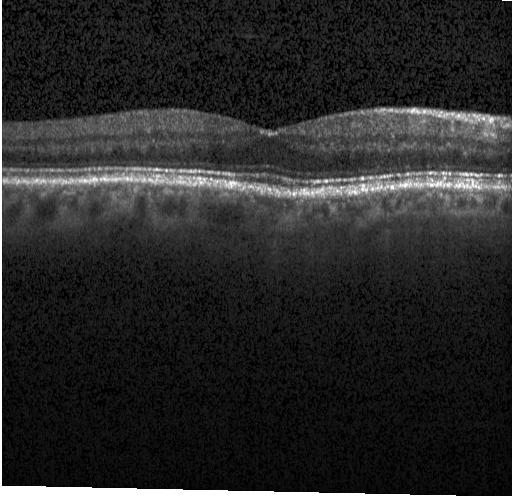 Heidelberg Spectralis, retinal OCT cross-section, centered on the fovea, spectral-domain OCT. Impression: no choroidal neovascularization, no diabetic macular edema, and no drusen.